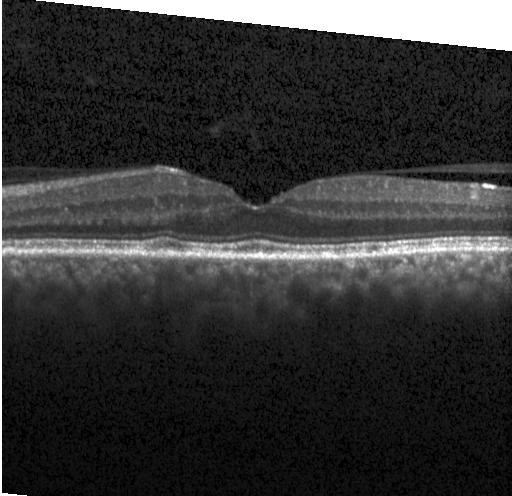

Assessment: multiple drusen.